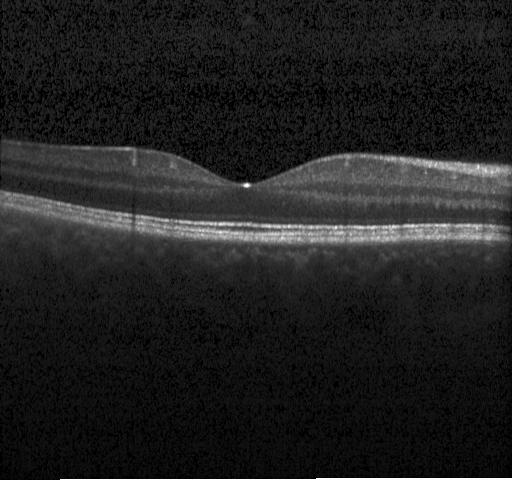

SD-OCT, optical coherence tomography scan, fovea-centered
Diagnosis: no evidence of CNV, DME, or drusen.